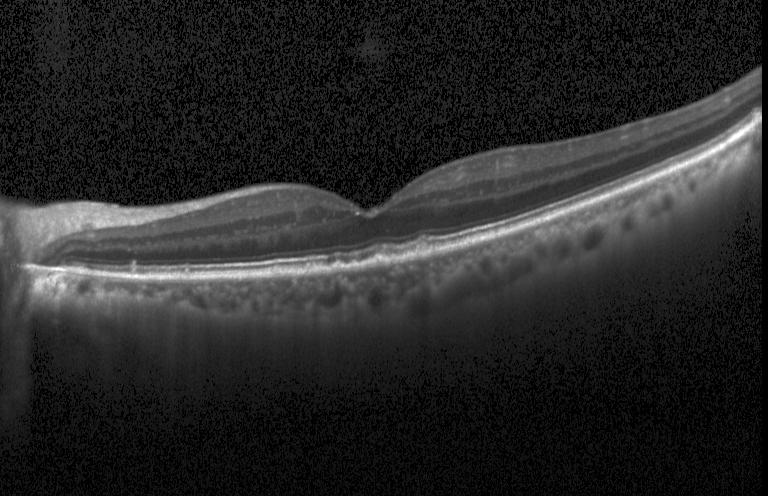

Through the macula, Heidelberg Spectralis, optical coherence tomography B-scan
Diagnosis: sub-RPE drusenoid deposits.